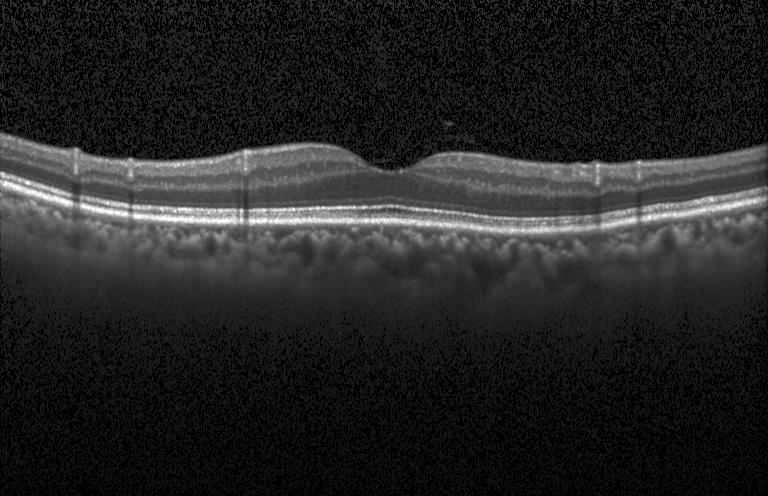 OCT finding: no choroidal neovascularization, no diabetic macular edema, and no drusen.